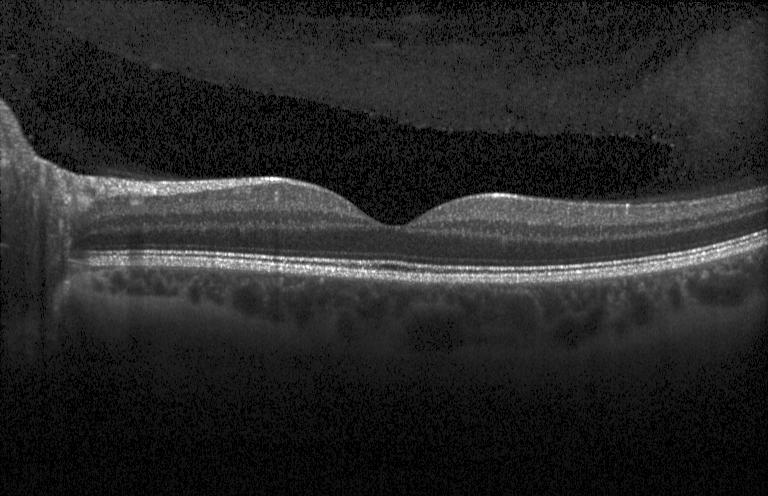 OCT B-scan showing no evidence of choroidal neovascularization, diabetic macular edema, or drusen.